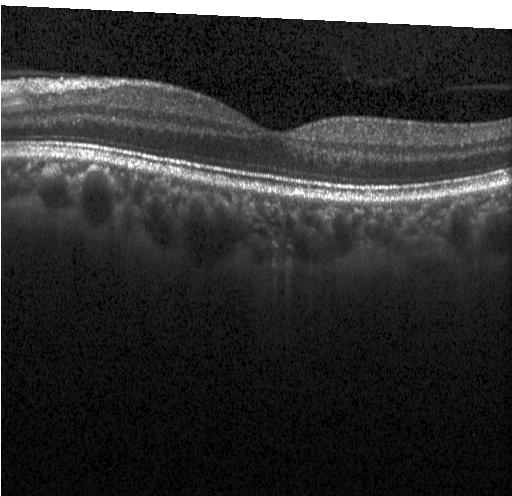 Horizontal scan through the fovea. Spectral-domain optical coherence tomography. OCT line scan — Diagnosis: no choroidal neovascularization, no diabetic macular edema, and no drusen.